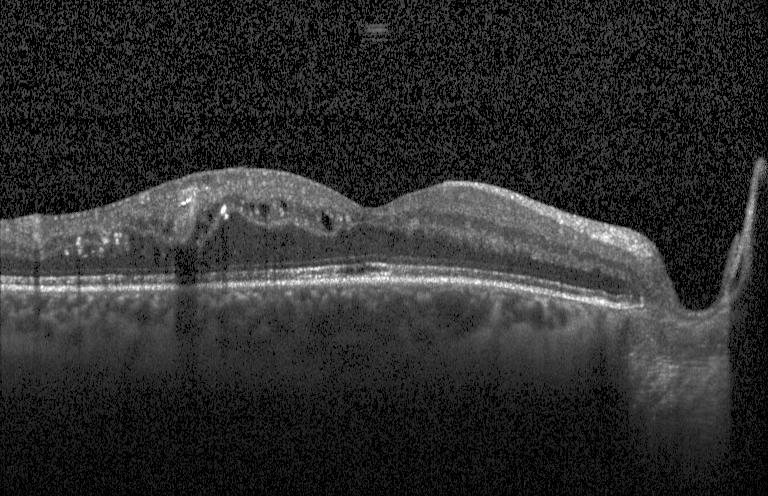 Retinal OCT cross-section showing diabetic macular edema (DME).